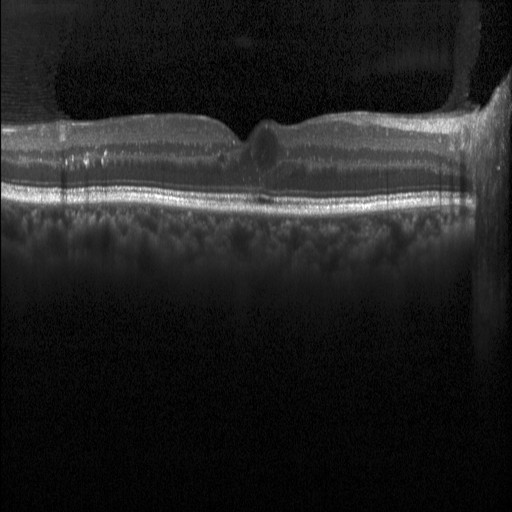

Diabetic macular edema.